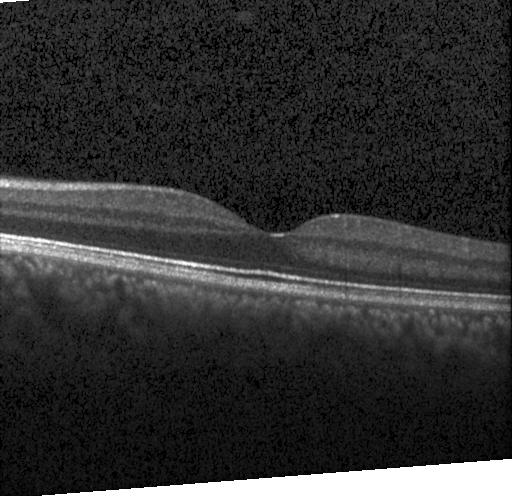

Heidelberg Spectralis OCT system. Through the macula. OCT B-scan
Finding: no choroidal neovascularization, no diabetic macular edema, and no drusen.